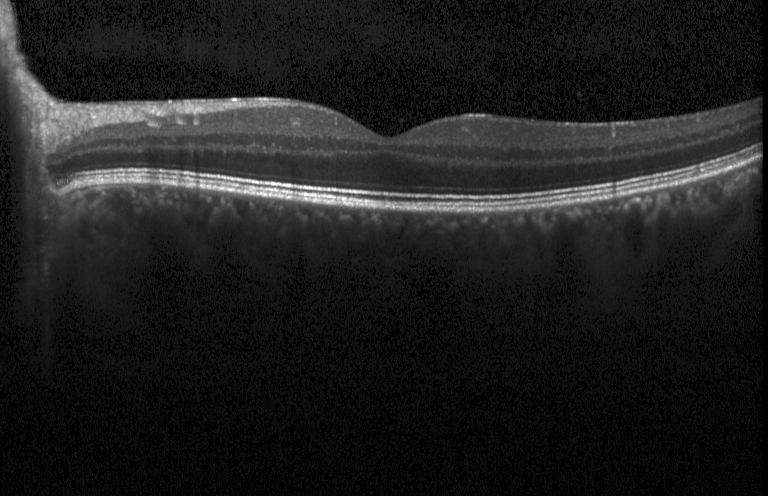 Spectral-domain optical coherence tomography, through the macula, Heidelberg Spectralis, retinal OCT B-scan
This B-scan demonstrates no choroidal neovascularization, diabetic macular edema, or drusen.